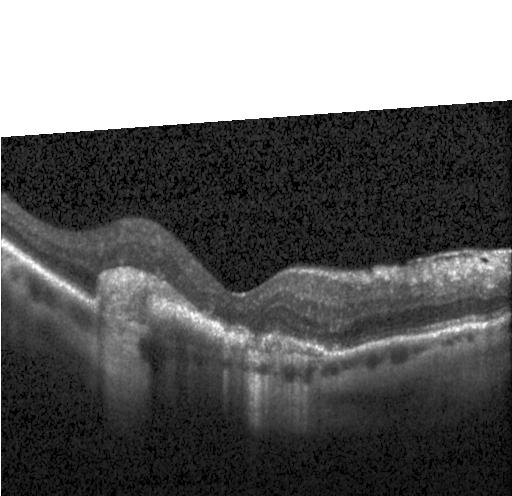 Optical coherence tomography scan
Choroidal neovascularization.